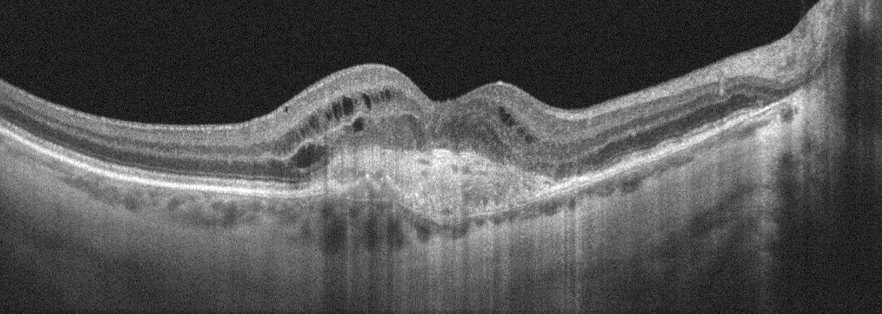

OCT B-scan
This B-scan demonstrates age-related macular degeneration (AMD).